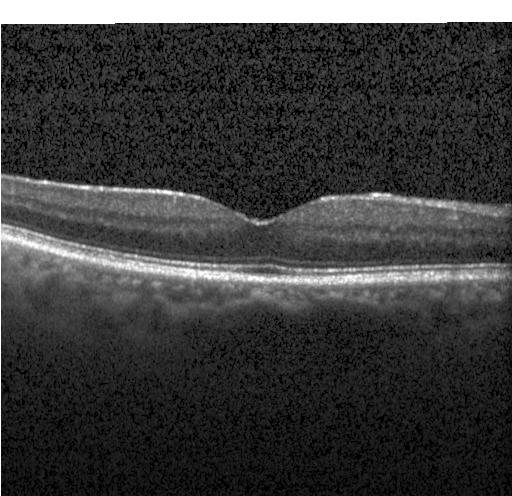 OCT B-scan, through the macula — Finding: no evidence of choroidal neovascularization, diabetic macular edema, or drusen.